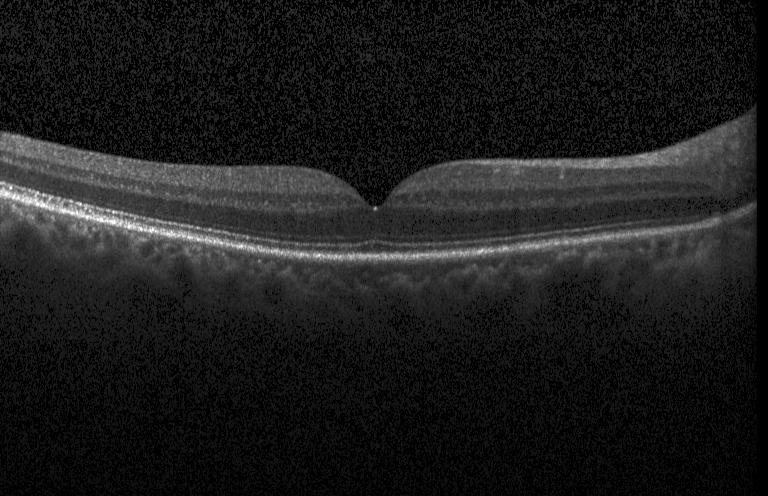

OCT B-scan. SD-OCT. Heidelberg Spectralis — Diagnosis: no evidence of CNV, DME, or drusen.